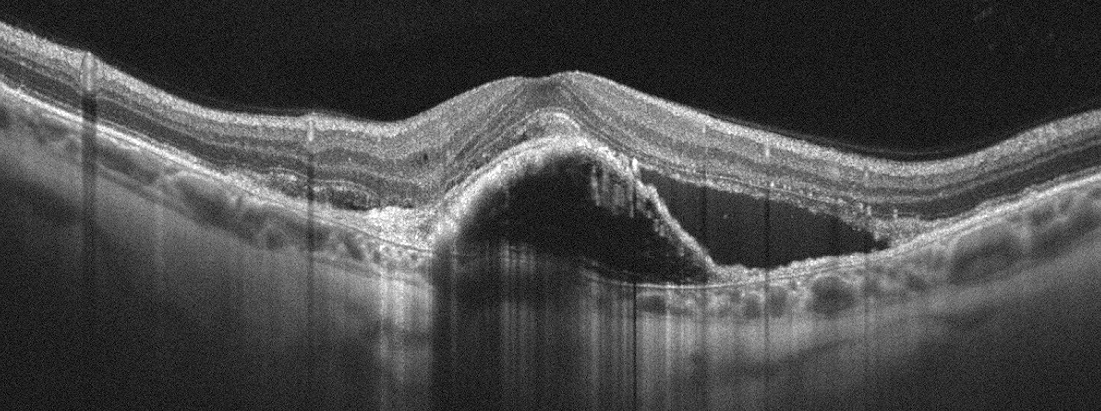 Diagnosis: age-related macular degeneration (AMD).